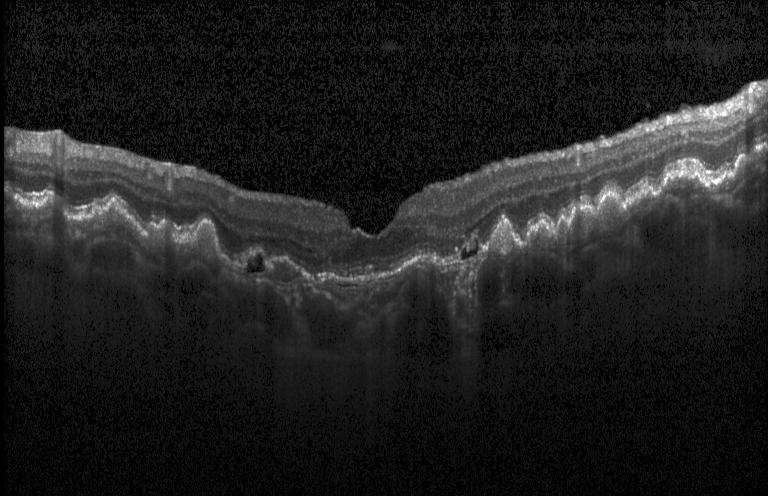
Retinal OCT B-scan. Dx: choroidal neovascularization (CNV).